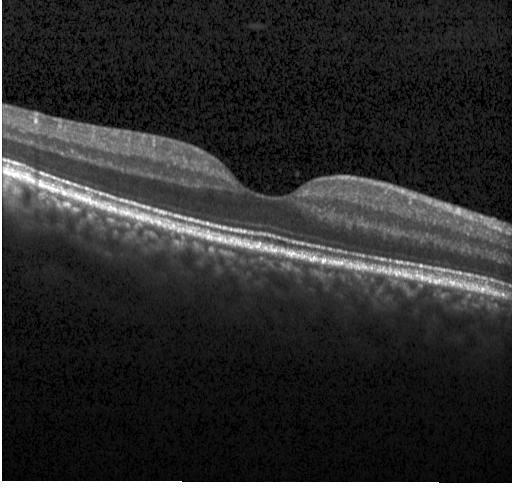 OCT finding: neither CNV, DME, nor drusen.